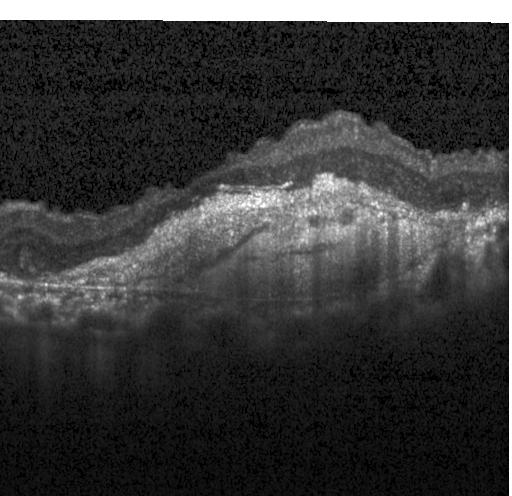 Finding: a choroidal neovascular membrane.